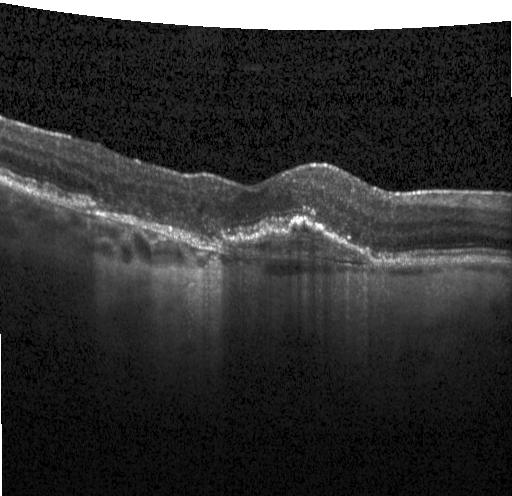 Heidelberg Spectralis; optical coherence tomography scan; SD-OCT; horizontal scan through the fovea. Choroidal neovascularization (CNV).